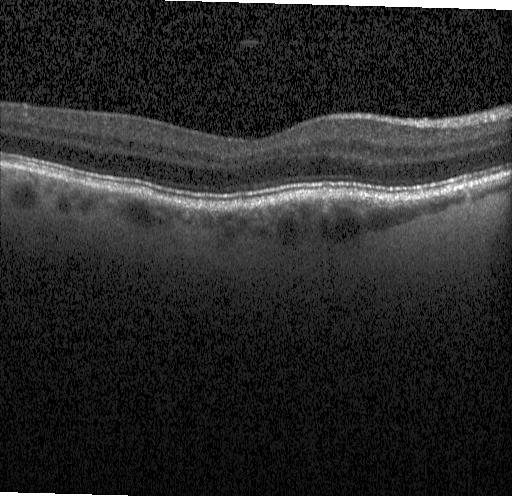

Instrument: Heidelberg Spectralis. Retinal OCT B-scan — Diagnosis: no evidence of choroidal neovascularization, diabetic macular edema, or drusen.